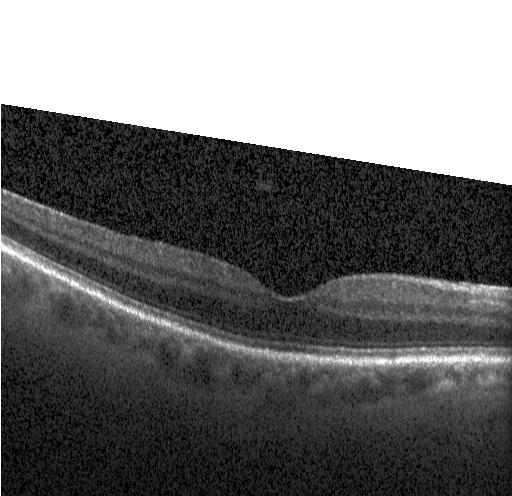 Impression: no CNV, DME, or drusen.